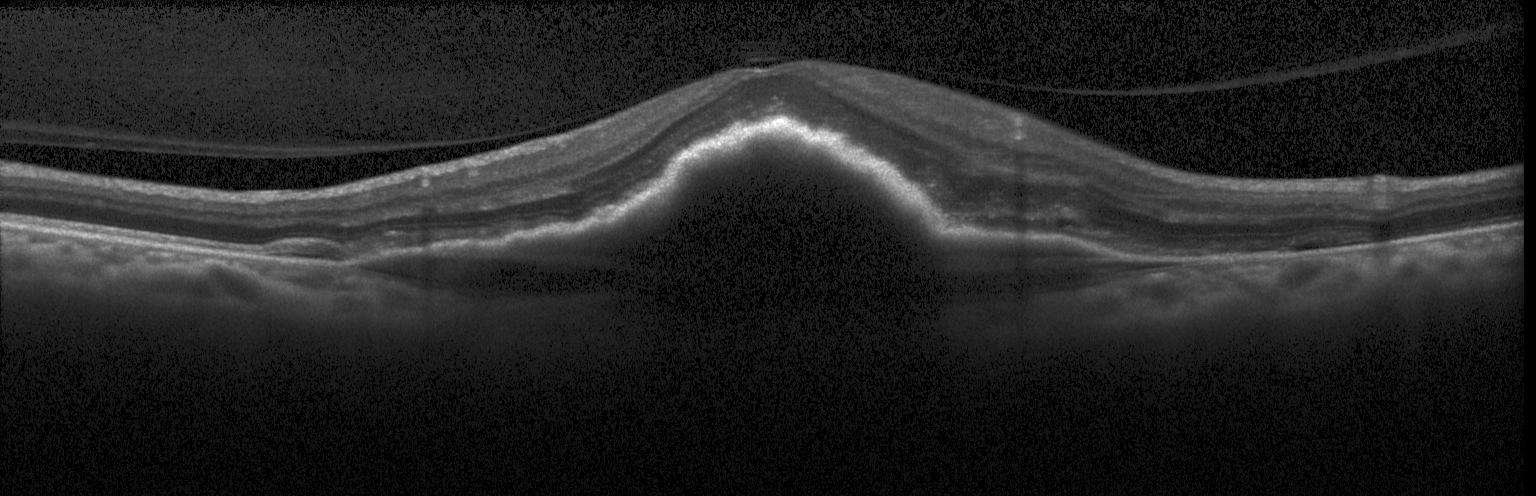
Assessment: choroidal neovascularization (CNV).